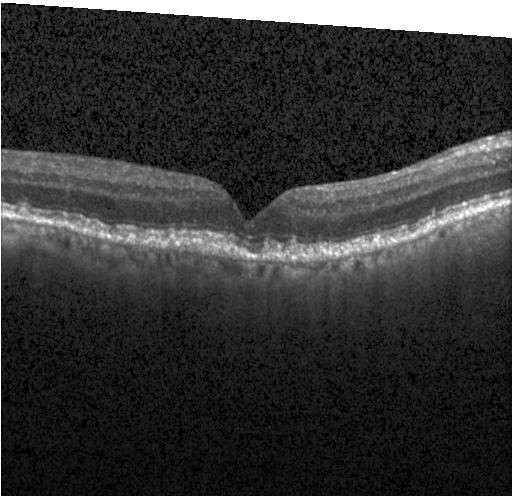
Dx: drusen.